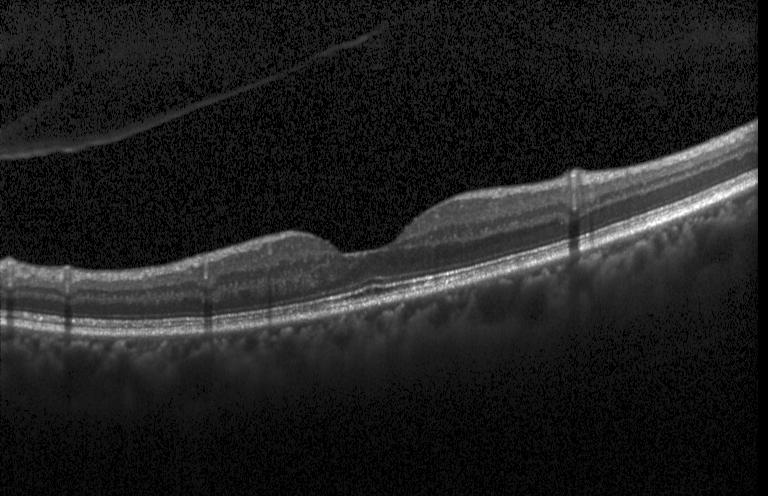
Optical coherence tomography scan. Spectral-domain OCT. Heidelberg Spectralis.
Macular OCT: no choroidal neovascularization, diabetic macular edema, or drusen.